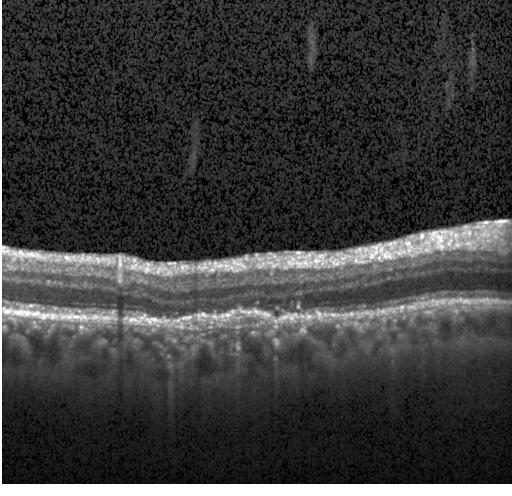
The scan shows choroidal neovascularization.